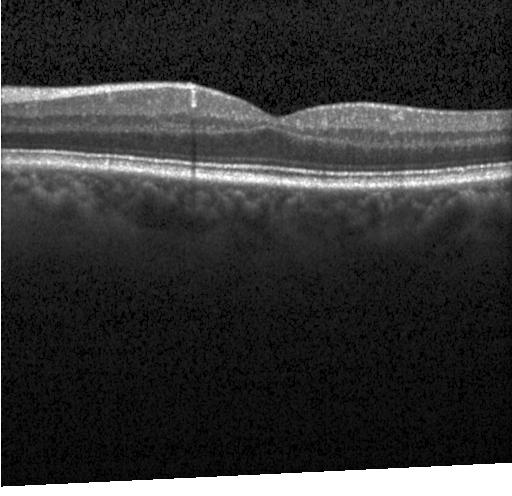
The scan shows no choroidal neovascularization, no diabetic macular edema, and no drusen.